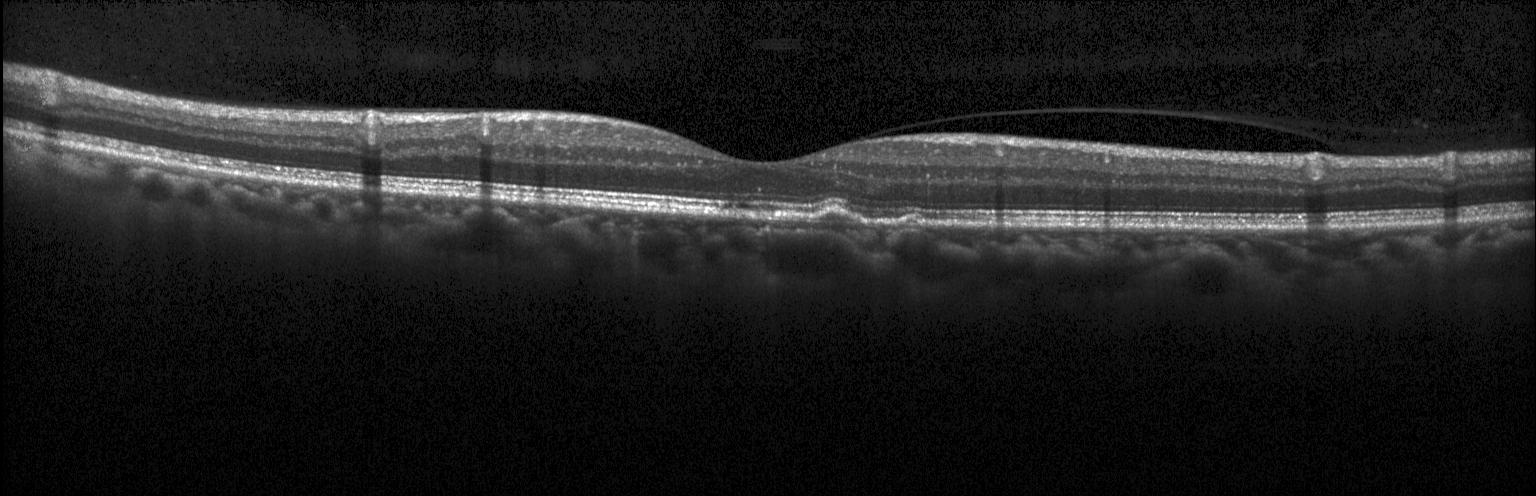
Macular scan · optical coherence tomography scan.
Macular OCT: multiple drusen.